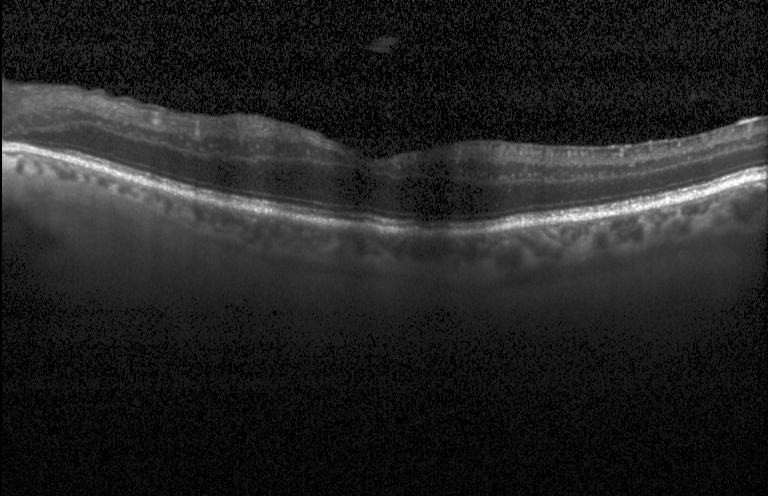
No choroidal neovascularization, diabetic macular edema, or drusen.